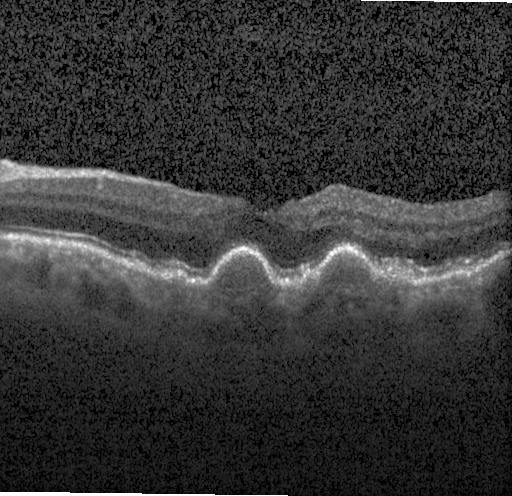
Impression: sub-RPE drusenoid deposits.